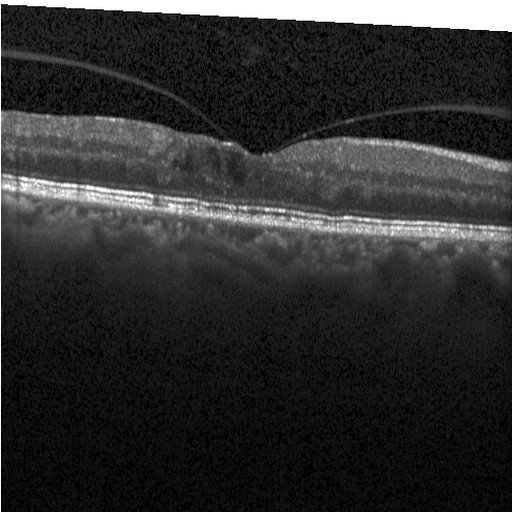 Retinal OCT cross-section showing diabetic macular edema.